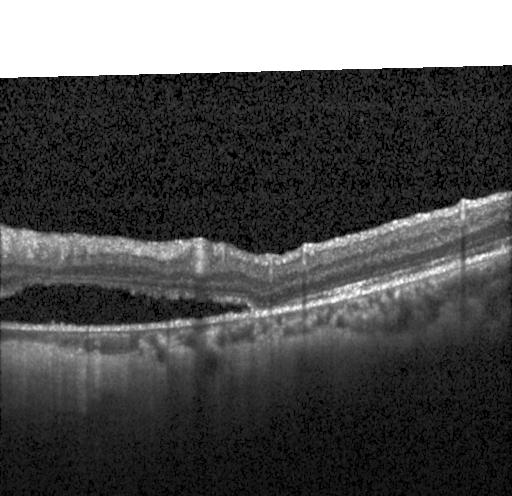 Acquired on a Heidelberg Spectralis; macular scan; optical coherence tomography B-scan; spectral-domain optical coherence tomography.
Finding: choroidal neovascularization (CNV).